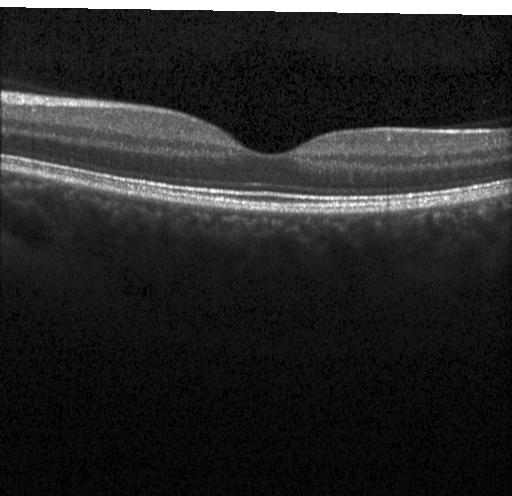 Optical coherence tomography scan. Diagnosis: no CNV, DME, or drusen.